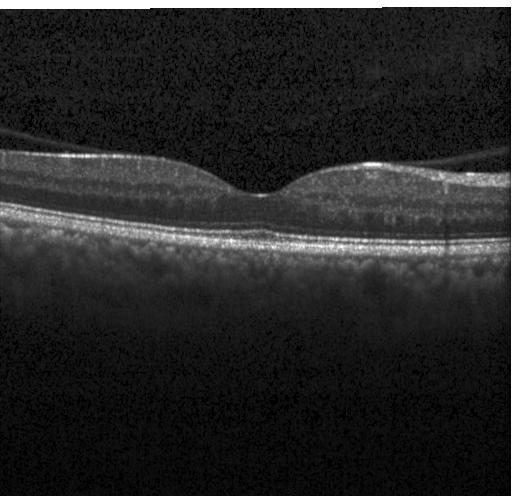

Macular scan · SD-OCT · retinal OCT B-scan · acquired on a Heidelberg Spectralis. Finding: no CNV, DME, or drusen.